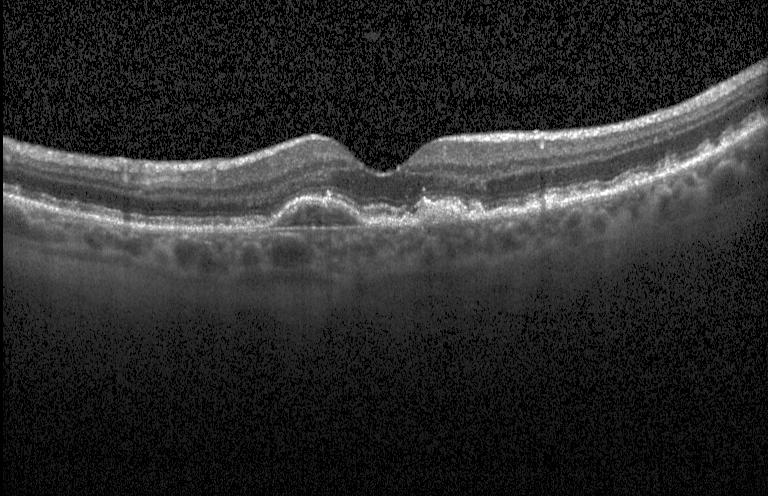 Spectral-domain OCT B-scan: choroidal neovascularization.